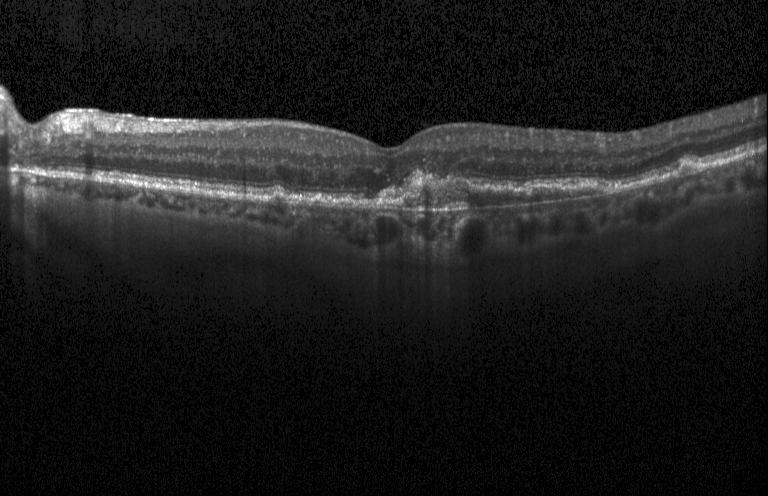 Spectral-domain optical coherence tomography · centered on the fovea · optical coherence tomography scan — CNV.